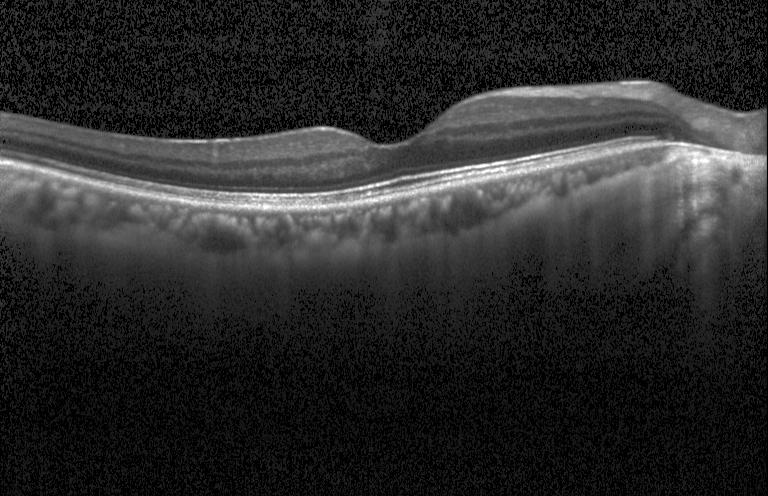
OCT finding: no evidence of choroidal neovascularization, diabetic macular edema, or drusen.